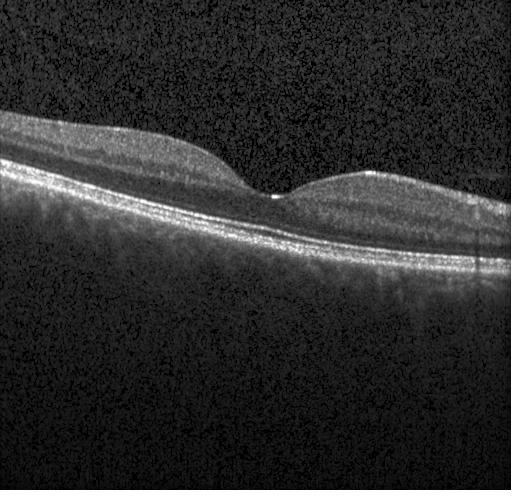 Centered on the fovea; optical coherence tomography scan; spectral-domain OCT; acquired on a Heidelberg Spectralis.
Finding: no evidence of choroidal neovascularization, diabetic macular edema, or drusen.